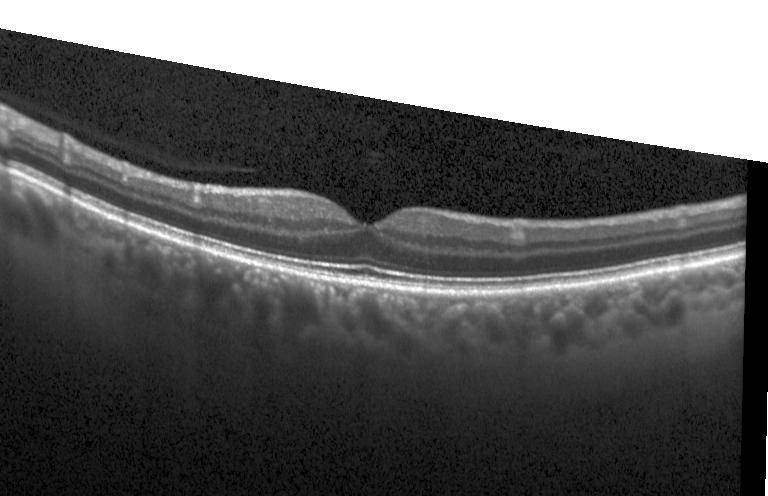 This B-scan demonstrates no CNV, no DME, and no drusen.